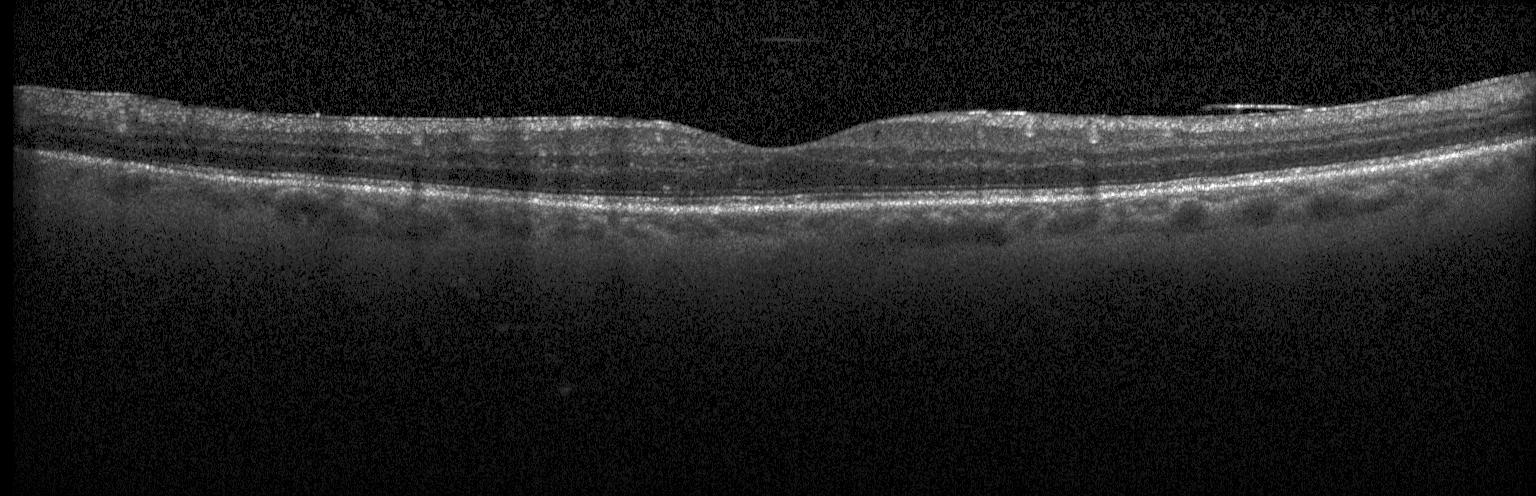
Optical coherence tomography B-scan; through the macula
This B-scan demonstrates neither choroidal neovascularization, diabetic macular edema, nor drusen.